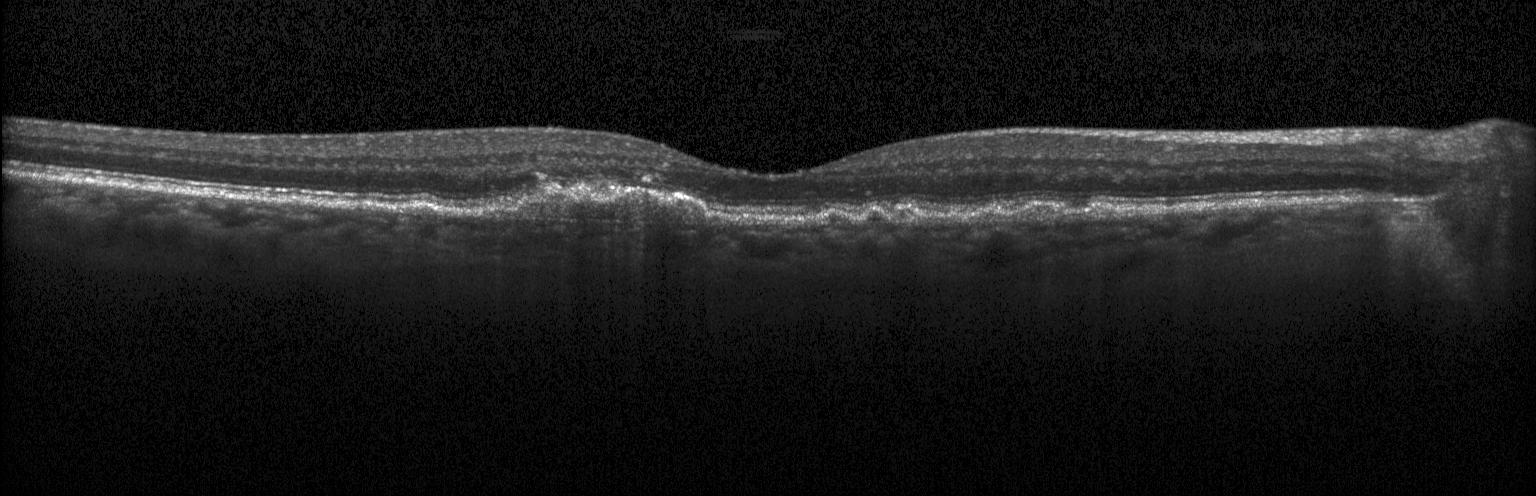

Acquired on a Heidelberg Spectralis · OCT line scan — This B-scan demonstrates a choroidal neovascular membrane.